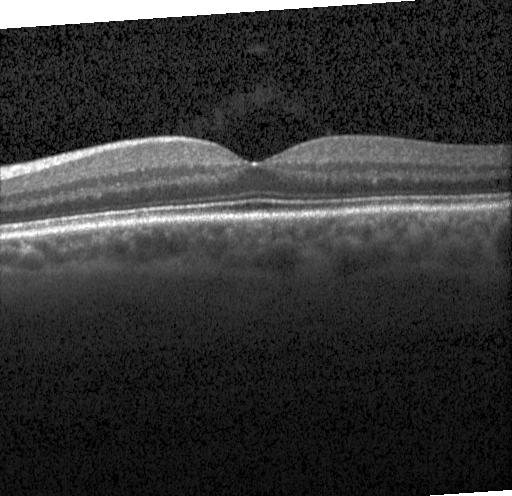

Heidelberg Spectralis OCT system · centered on the fovea · OCT B-scan · spectral-domain OCT
Diagnosis: neither CNV, DME, nor drusen.